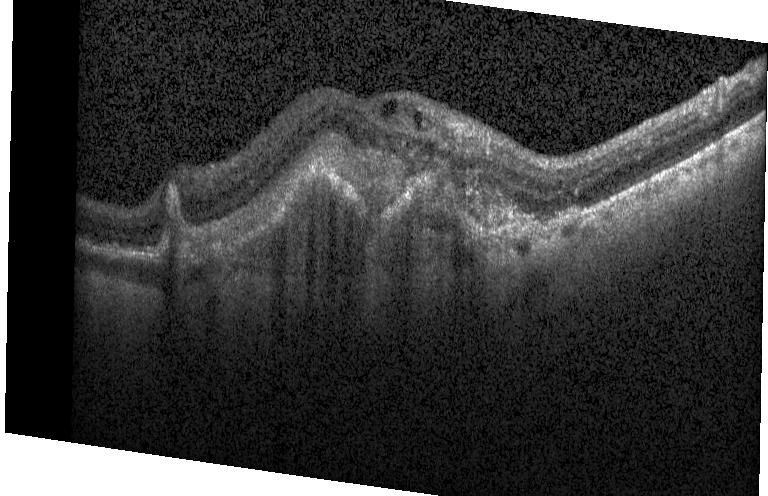
Macular OCT: CNV.